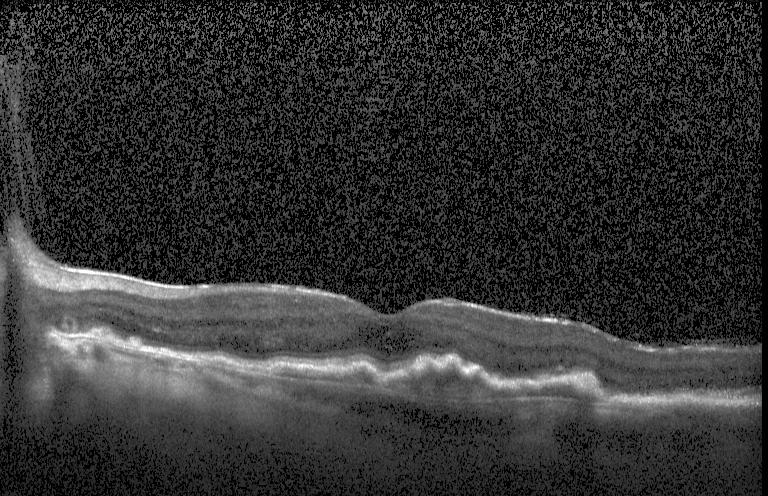 Retinal OCT B-scan.
Finding: CNV.